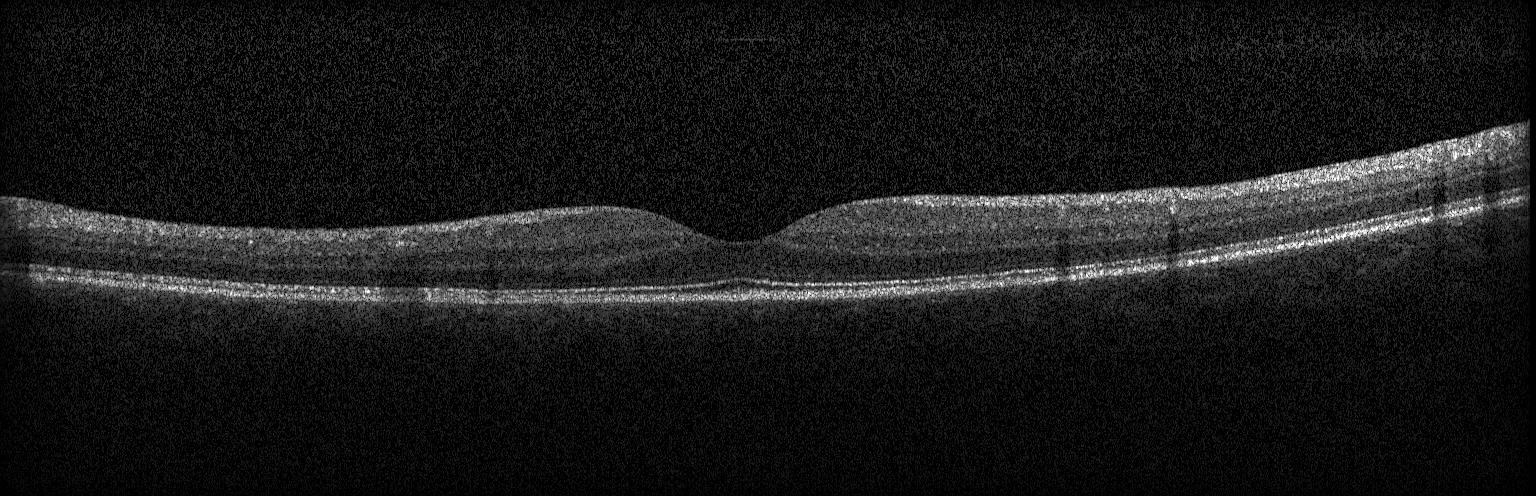 Heidelberg Spectralis OCT system · retinal OCT B-scan · spectral-domain OCT.
Impression: no CNV, no DME, and no drusen.